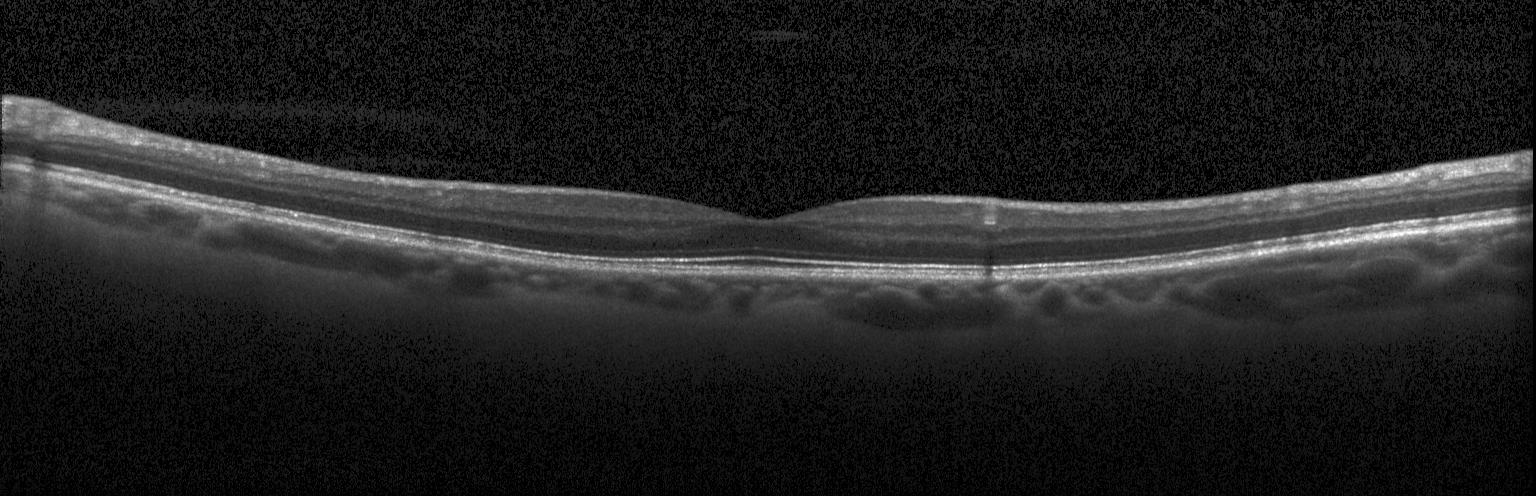 OCT B-scan showing neither choroidal neovascularization, diabetic macular edema, nor drusen.